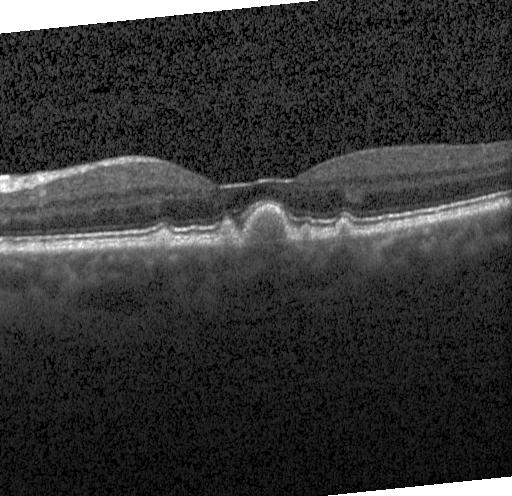

Centered on the fovea, instrument: Heidelberg Spectralis, optical coherence tomography B-scan. Dx: drusen.